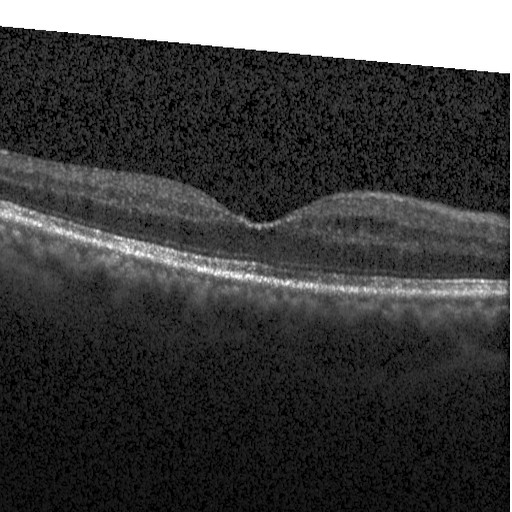

OCT B-scan showing DME.